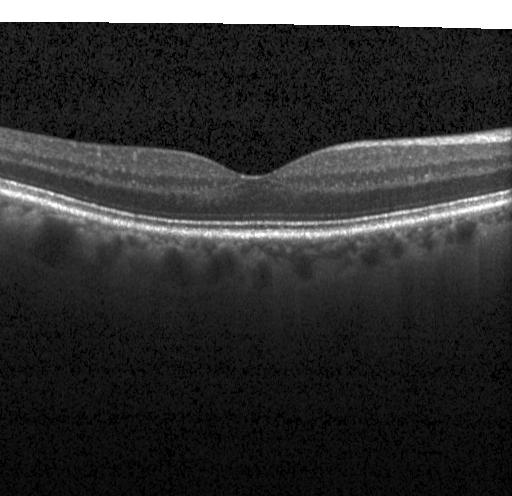
Diagnosis: no choroidal neovascularization, no diabetic macular edema, and no drusen.